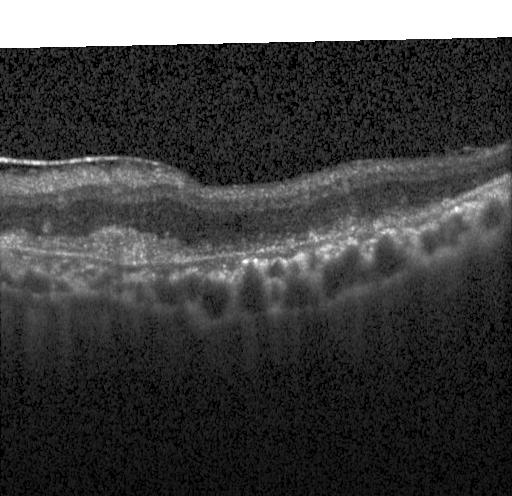 Assessment: a choroidal neovascular membrane.